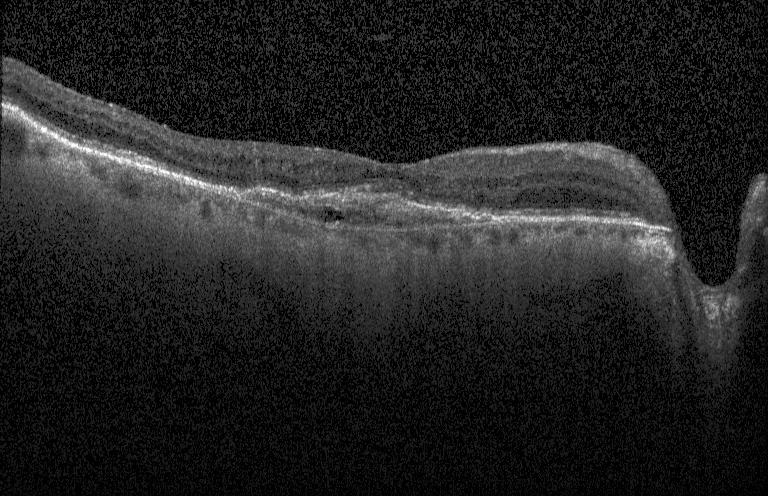
Retinal OCT B-scan
Finding: choroidal neovascularization.